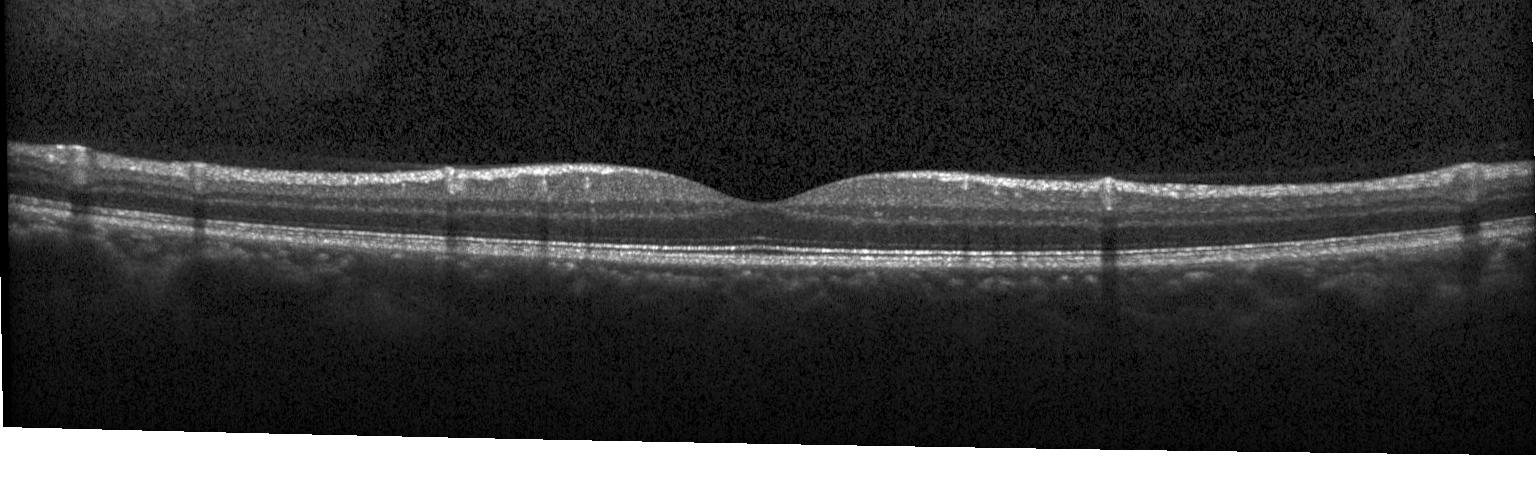

OCT line scan. Spectral-domain OCT — Dx: no CNV, DME, or drusen.